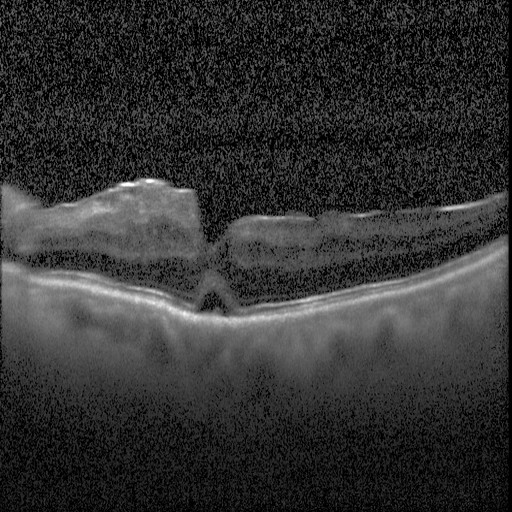 OCT finding: DME.